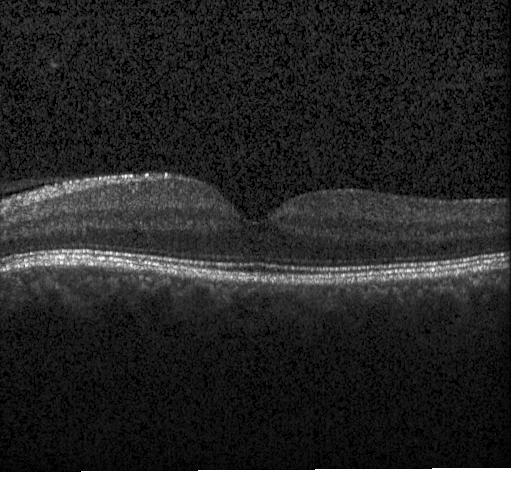 No choroidal neovascularization, no diabetic macular edema, and no drusen.